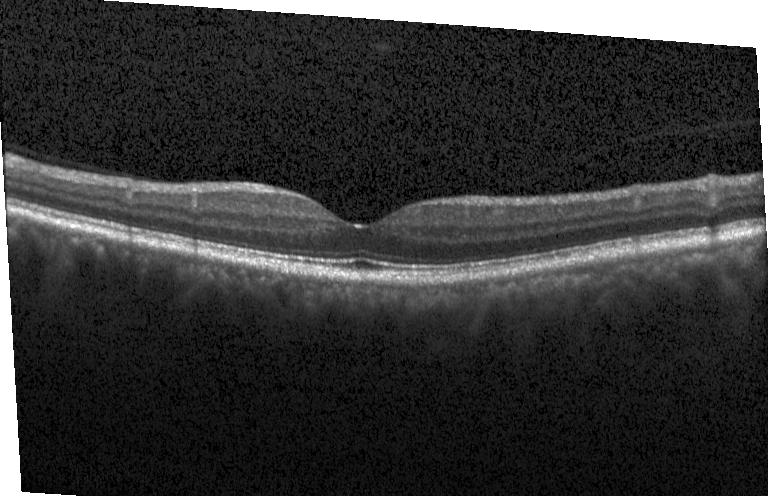

This B-scan demonstrates no evidence of CNV, DME, or drusen.